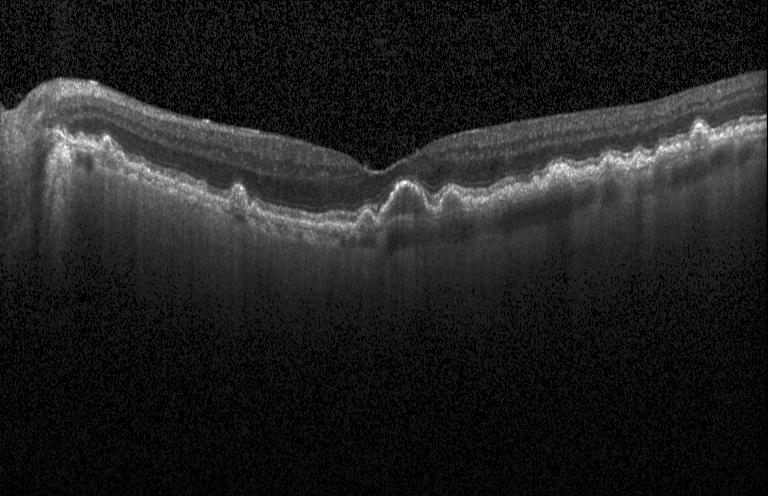 Spectral-domain OCT. Optical coherence tomography B-scan. Impression: multiple drusen.